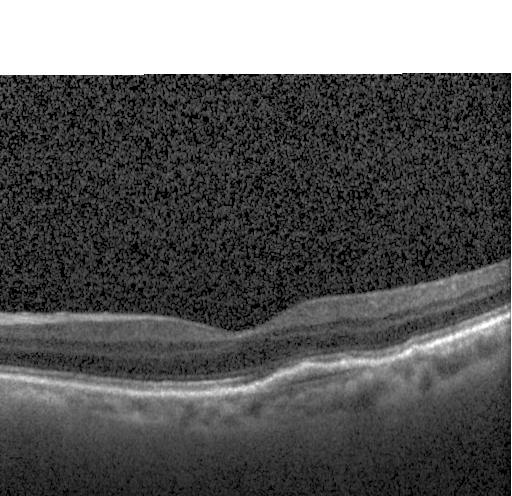

Optical coherence tomography scan; horizontal scan through the fovea; SD-OCT; Heidelberg Spectralis. Impression: choroidal neovascularization.